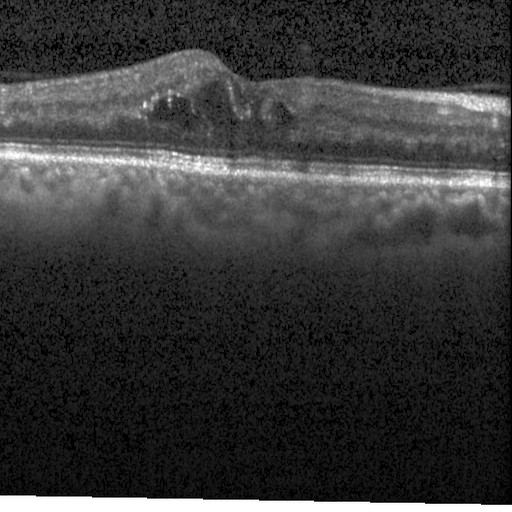
OCT line scan, spectral-domain optical coherence tomography.
Dx: DME.